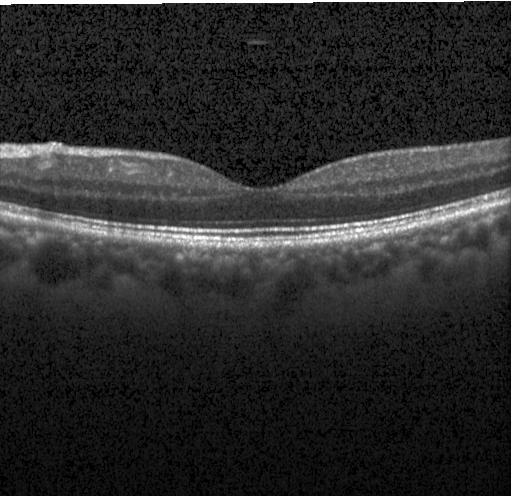
OCT B-scan. Spectral-domain OCT. Dx: neither choroidal neovascularization, diabetic macular edema, nor drusen.